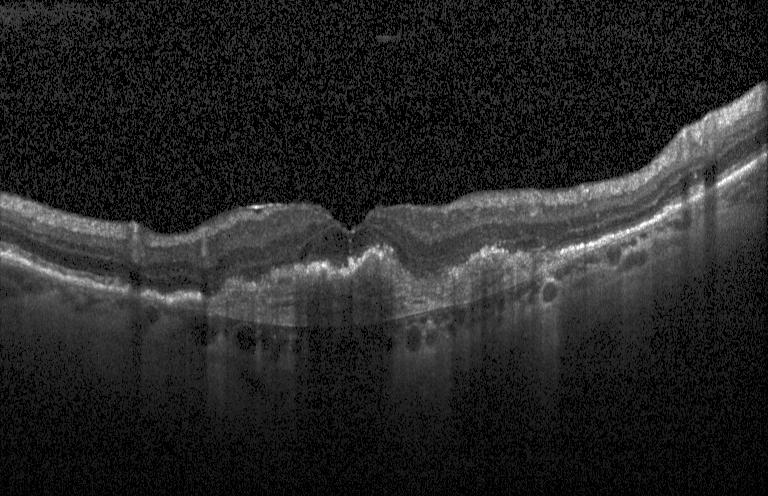
Retinal OCT cross-section, Heidelberg Spectralis.
Impression: a choroidal neovascular membrane.